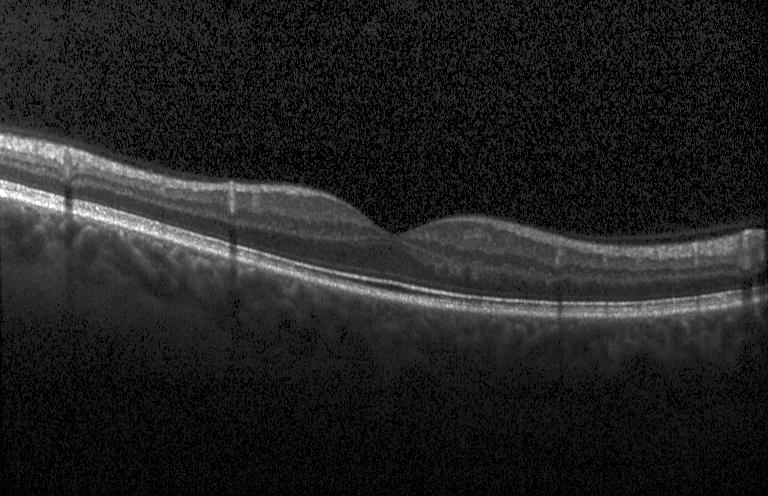 OCT scan showing neither choroidal neovascularization, diabetic macular edema, nor drusen.